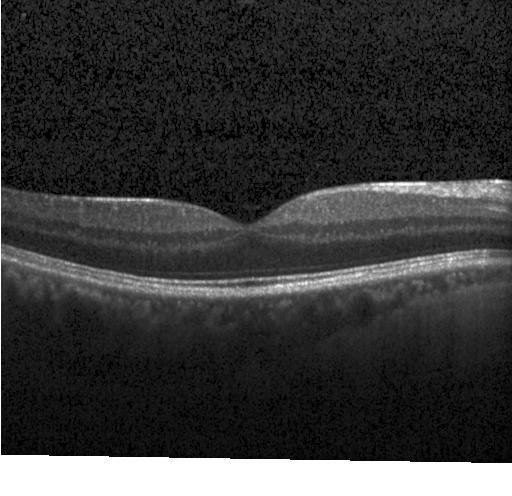
No evidence of choroidal neovascularization, diabetic macular edema, or drusen.